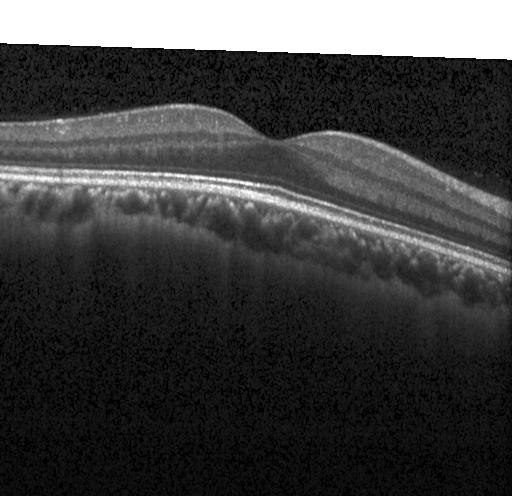
Retinal OCT B-scan
Finding: no choroidal neovascularization, no diabetic macular edema, and no drusen.